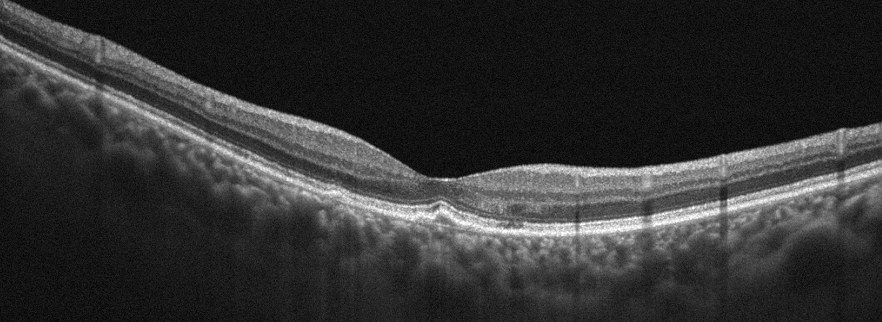
OCT B-scan showing AMD.